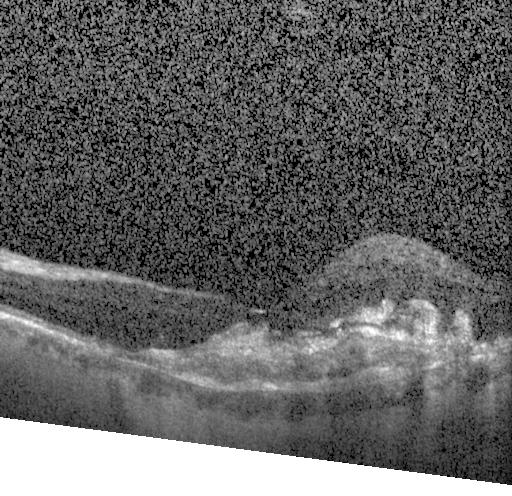

Through the macula, optical coherence tomography scan, Heidelberg Spectralis OCT system, spectral-domain OCT.
Impression: a choroidal neovascular membrane.